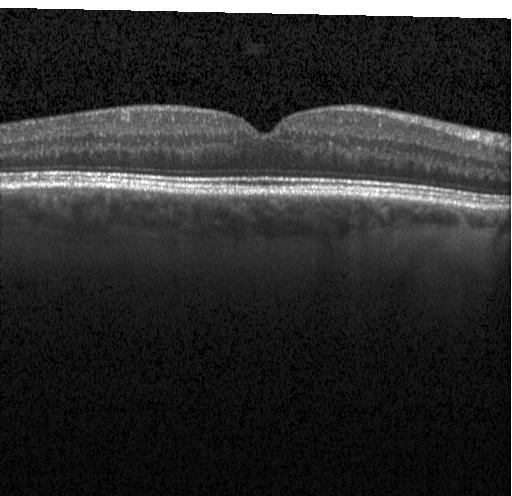
Centered on the fovea. Instrument: Heidelberg Spectralis. Retinal OCT cross-section.
This B-scan demonstrates no evidence of CNV, DME, or drusen.